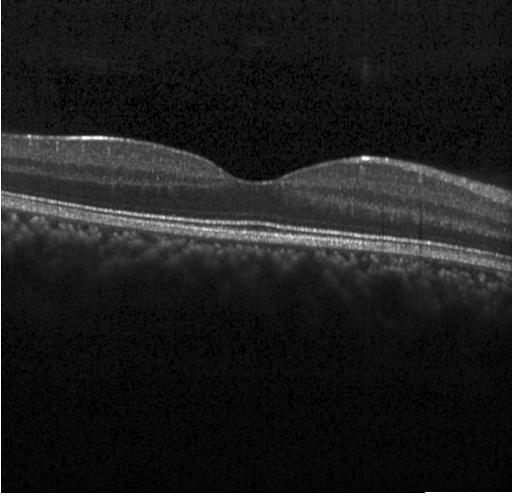

Heidelberg Spectralis; through the macula; OCT line scan — This B-scan demonstrates no evidence of choroidal neovascularization, diabetic macular edema, or drusen.